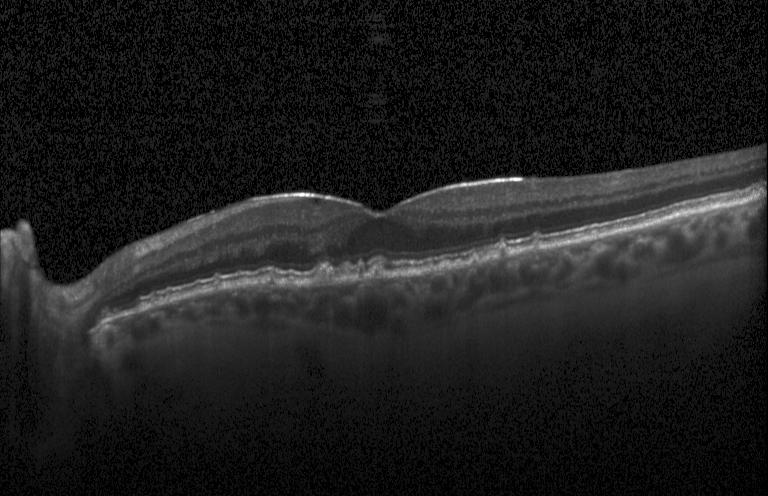
OCT B-scan showing multiple drusen.